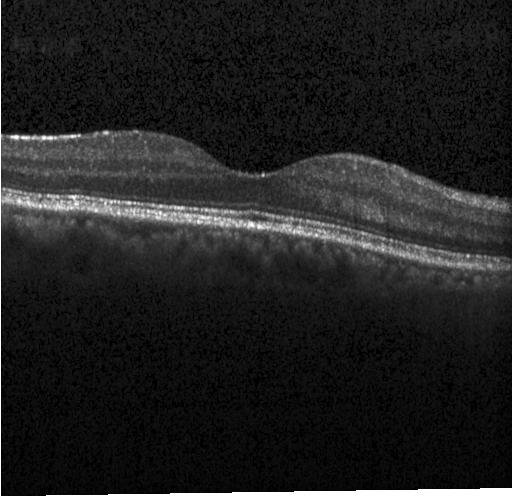
OCT B-scan showing no choroidal neovascularization, diabetic macular edema, or drusen.